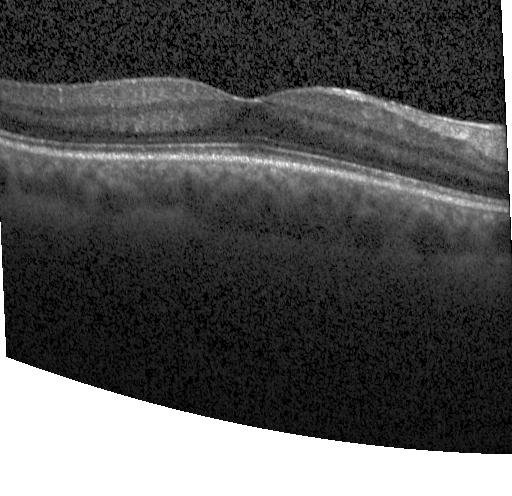

Retinal OCT B-scan · through the macula.
Impression: neither choroidal neovascularization, diabetic macular edema, nor drusen.